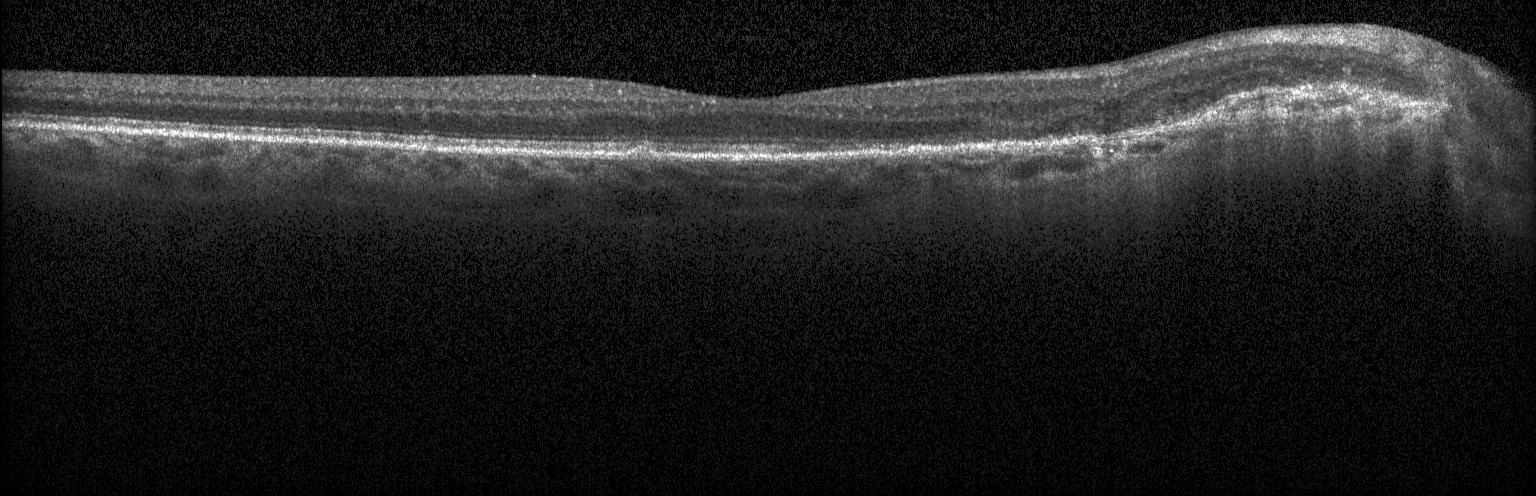

Impression: CNV.